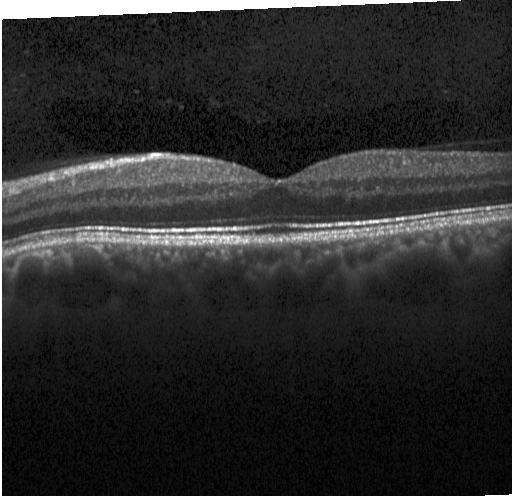 Finding: no choroidal neovascularization, no diabetic macular edema, and no drusen.